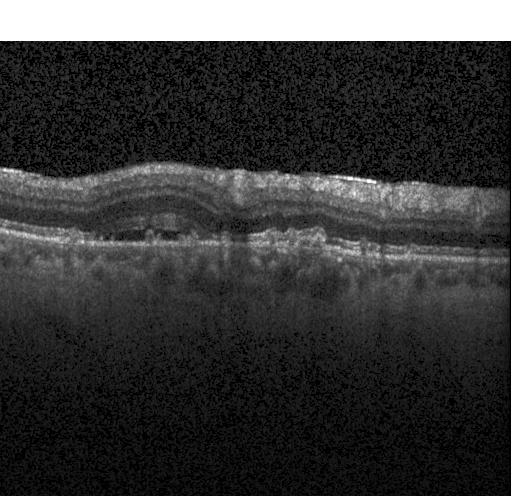

Retinal OCT cross-section. Assessment: a choroidal neovascular membrane.